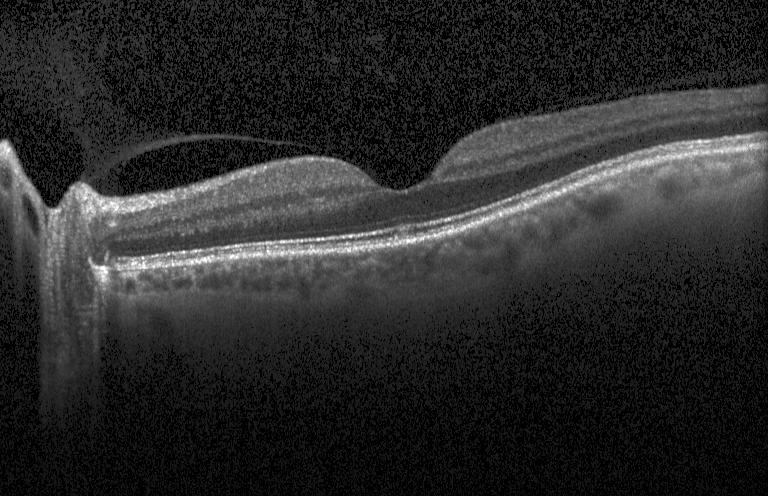

Diagnosis: neither CNV, DME, nor drusen.